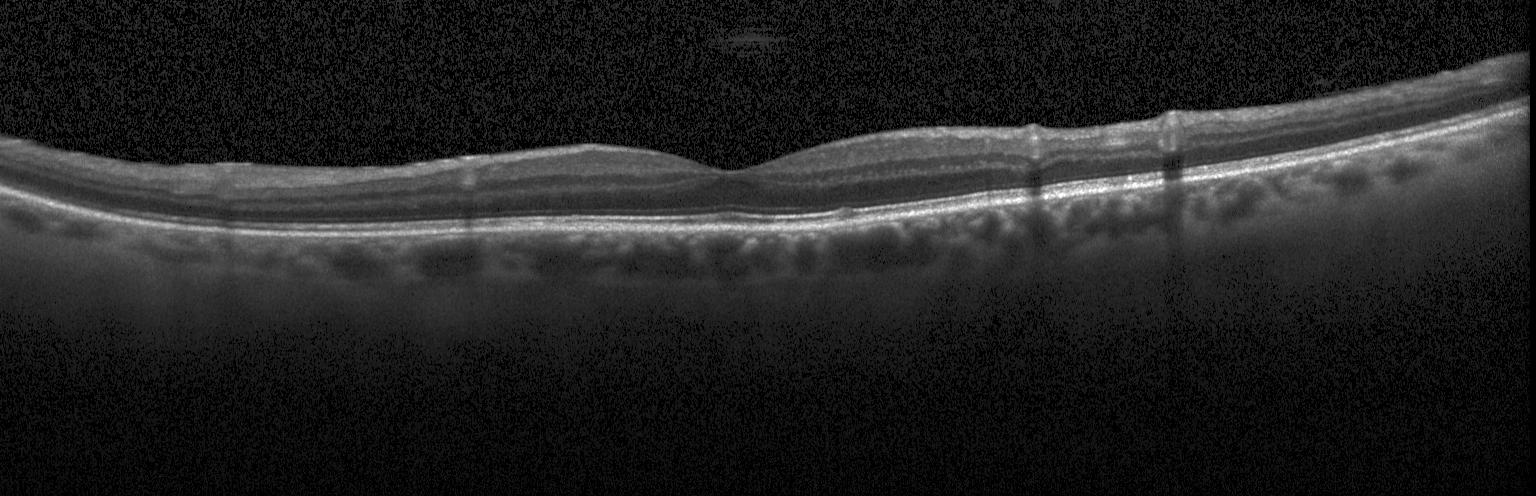 Macular scan, OCT line scan, instrument: Heidelberg Spectralis. Assessment: no choroidal neovascularization, diabetic macular edema, or drusen.